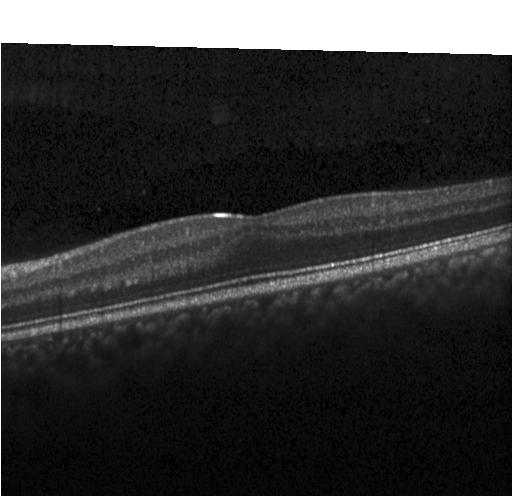 Retinal OCT cross-section showing no CNV, DME, or drusen.